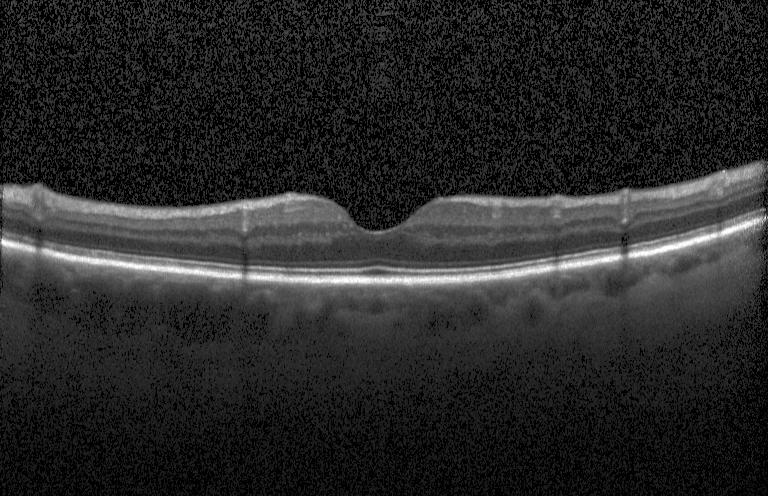

Finding: neither choroidal neovascularization, diabetic macular edema, nor drusen.